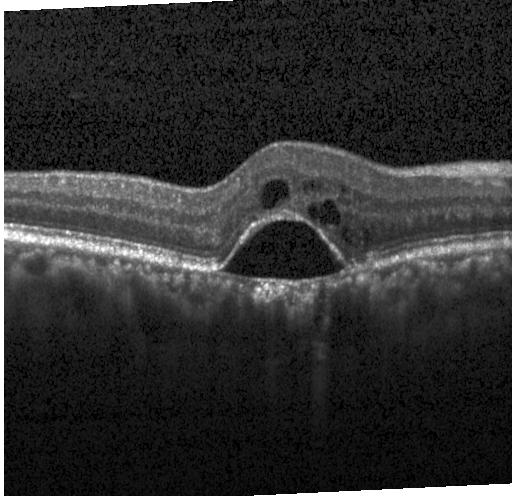

Optical coherence tomography scan. The scan shows a choroidal neovascular membrane.